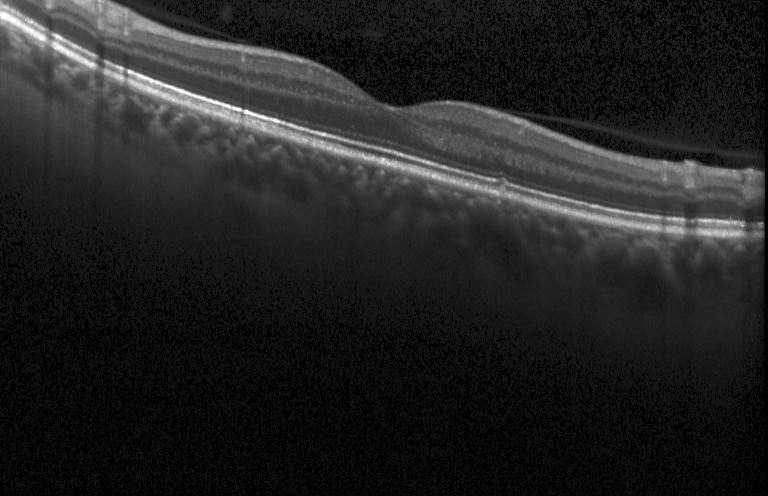
Retinal OCT cross-section, spectral-domain optical coherence tomography, acquired on a Heidelberg Spectralis
Finding: sub-RPE drusenoid deposits.